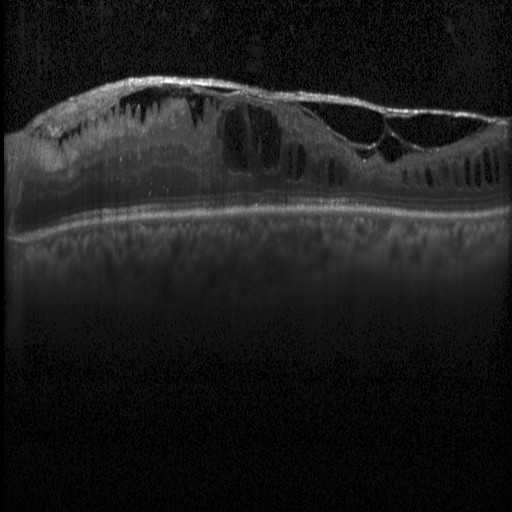
Spectral-domain OCT; through the macula; instrument: Heidelberg Spectralis; optical coherence tomography B-scan — Impression: DME.